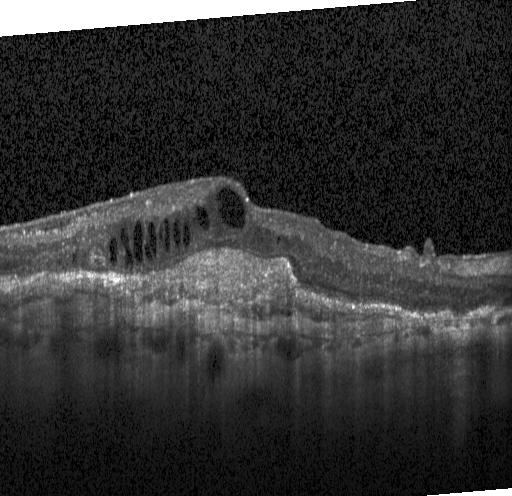
Spectral-domain OCT B-scan: CNV.